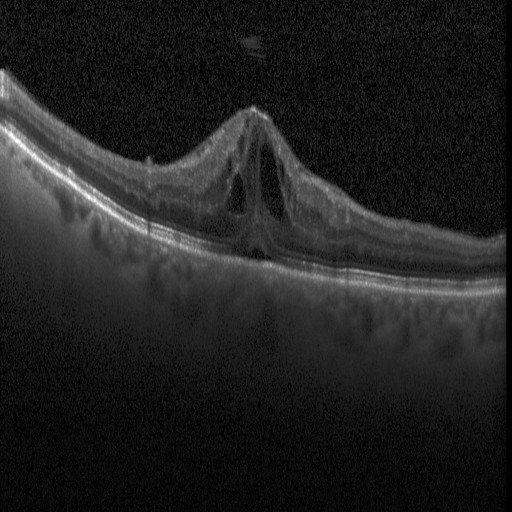 Spectral-domain optical coherence tomography. Macular scan. Retinal OCT B-scan. This B-scan demonstrates DME.